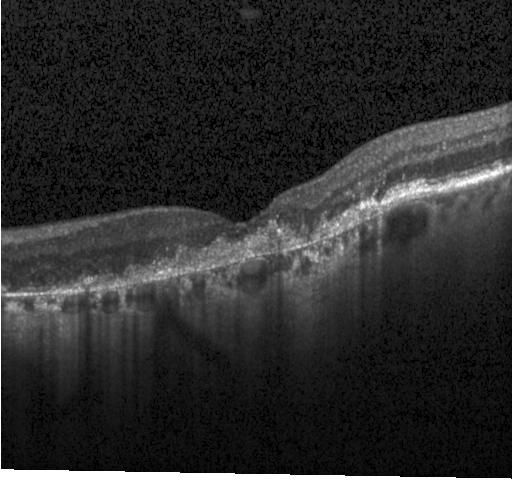 Heidelberg Spectralis. Centered on the fovea. Retinal OCT B-scan. Assessment: choroidal neovascularization.